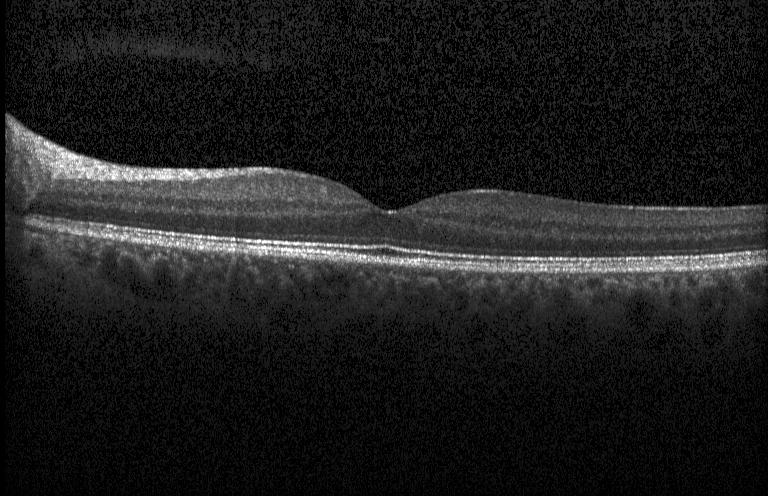 OCT finding: no CNV, DME, or drusen.